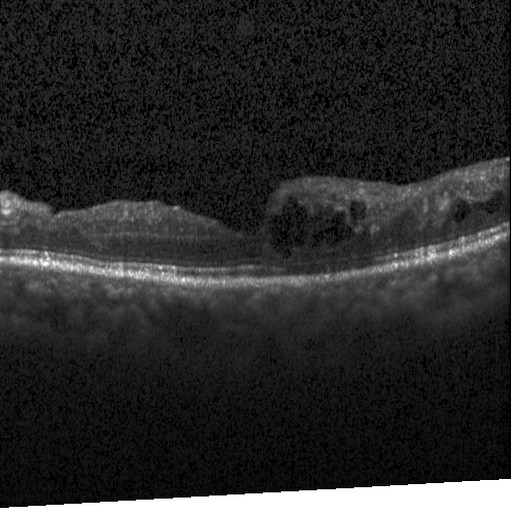

OCT finding: diabetic macular edema (DME).